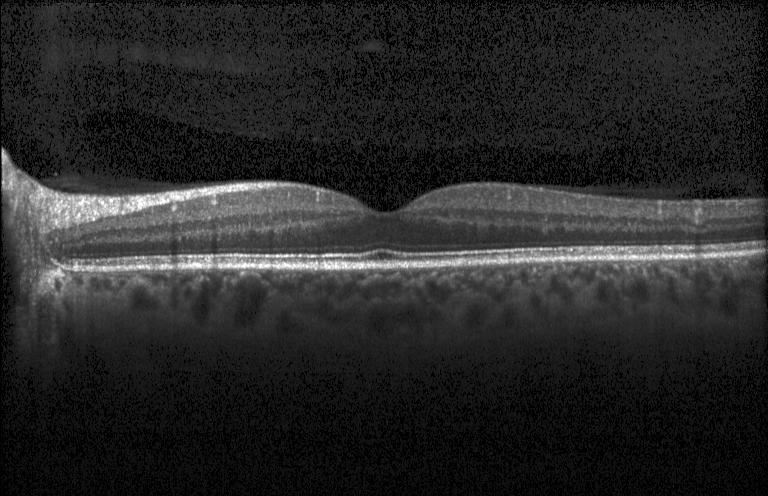
Spectral-domain OCT. OCT B-scan
Neither CNV, DME, nor drusen.